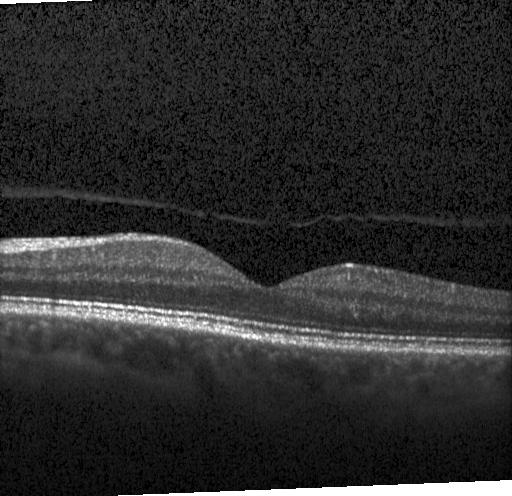
Diagnosis: no evidence of CNV, DME, or drusen.